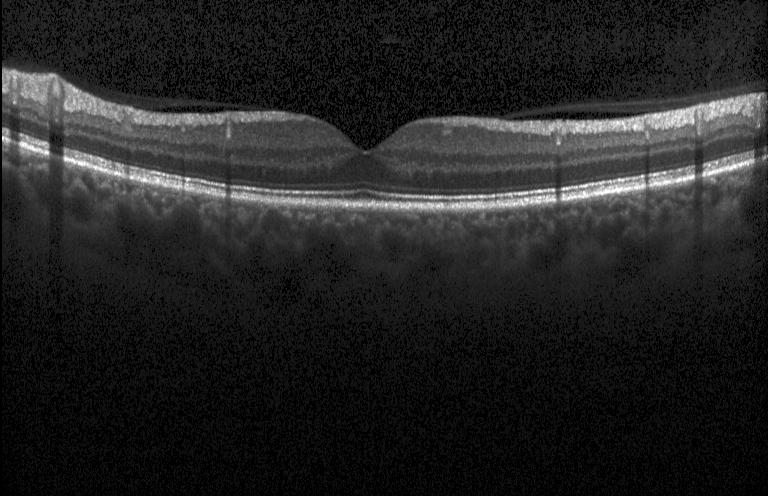
Through the macula · OCT B-scan · SD-OCT · Heidelberg Spectralis
Assessment: no CNV, no DME, and no drusen.